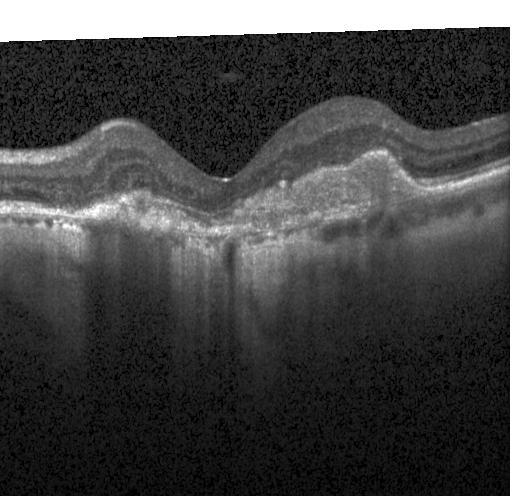

Through the macula. SD-OCT. Heidelberg Spectralis OCT system. Optical coherence tomography scan — This B-scan demonstrates CNV.